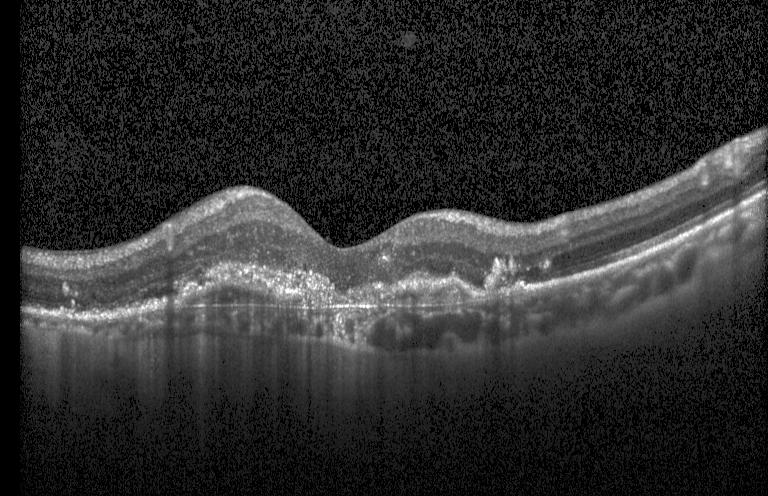

Fovea-centered; OCT B-scan; Heidelberg Spectralis; spectral-domain optical coherence tomography — Macular OCT: choroidal neovascularization.